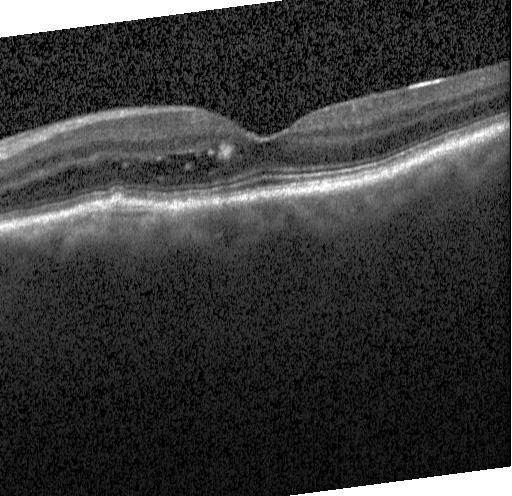

OCT finding: diabetic macular edema.